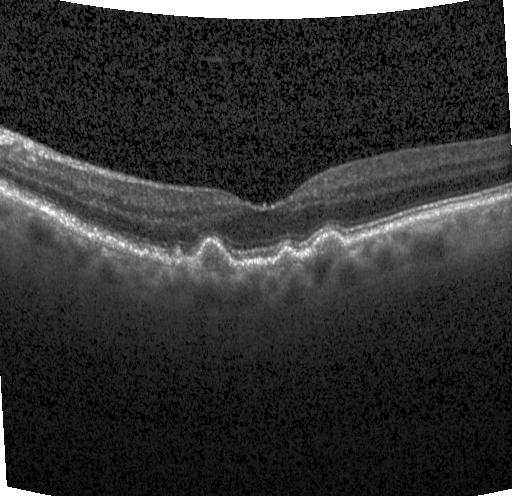

Instrument: Heidelberg Spectralis; retinal OCT cross-section; through the macula; SD-OCT. Impression: sub-RPE drusenoid deposits.